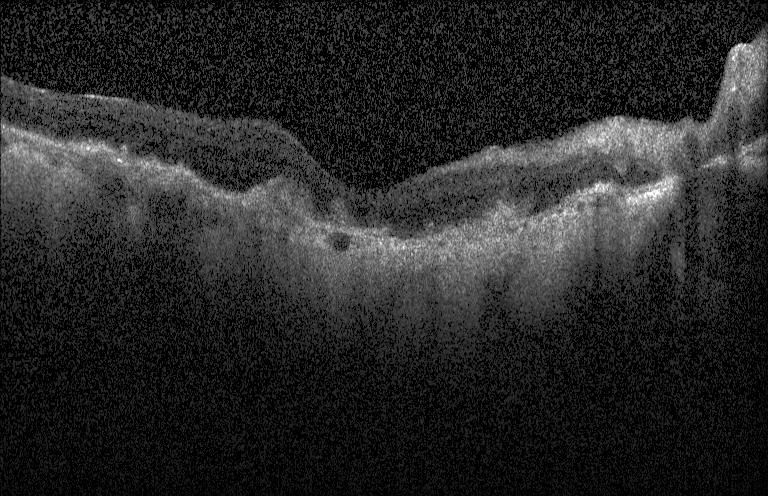
Retinal OCT cross-section showing choroidal neovascularization.